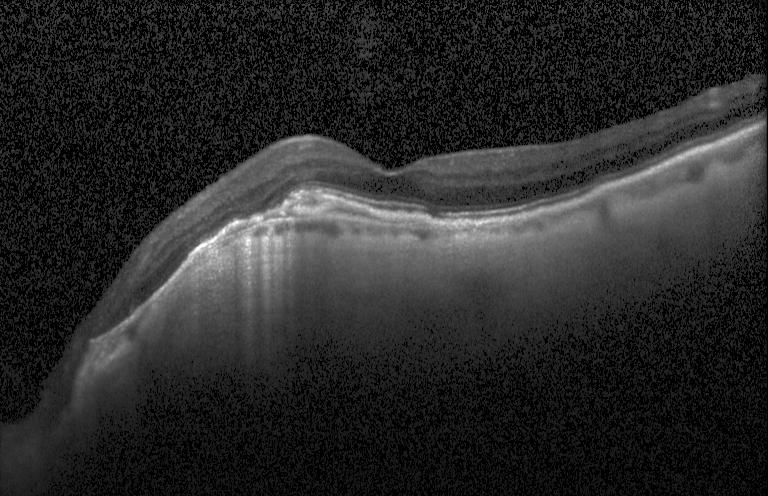 This B-scan demonstrates choroidal neovascularization.